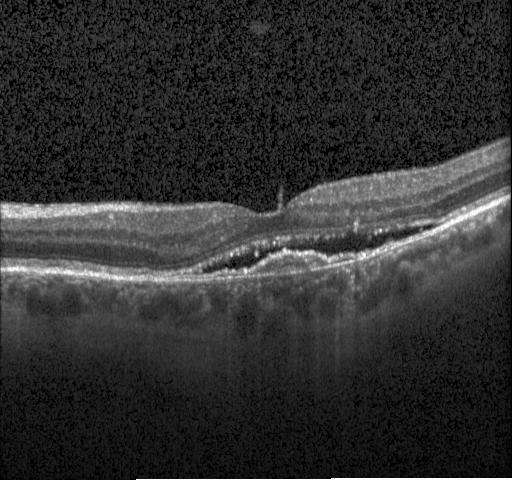

Impression: a choroidal neovascular membrane.